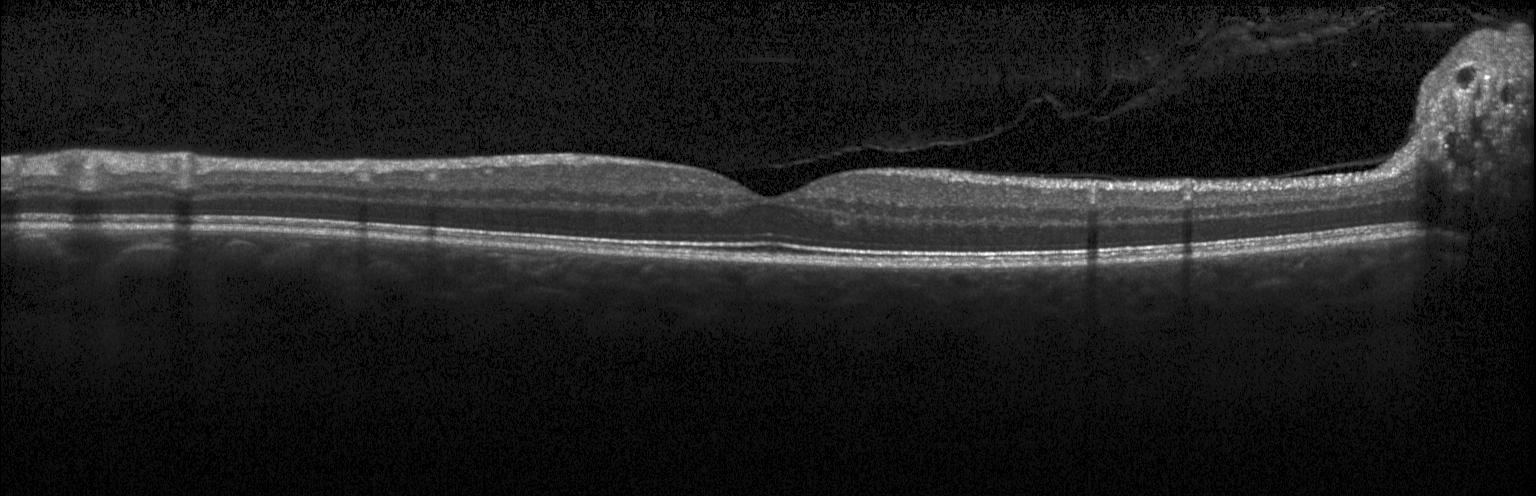 OCT B-scan — No CNV, DME, or drusen.